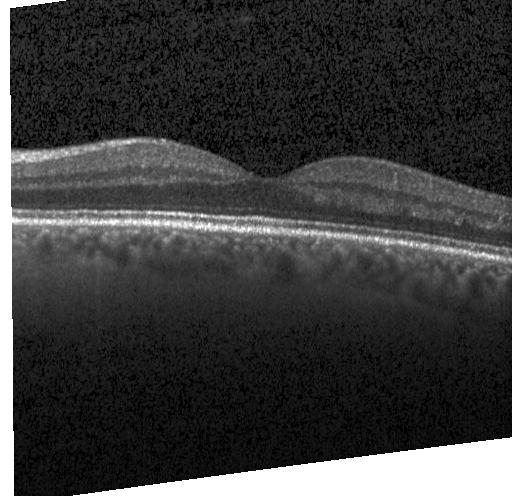
Horizontal scan through the fovea; optical coherence tomography scan — Diagnosis: no choroidal neovascularization, diabetic macular edema, or drusen.